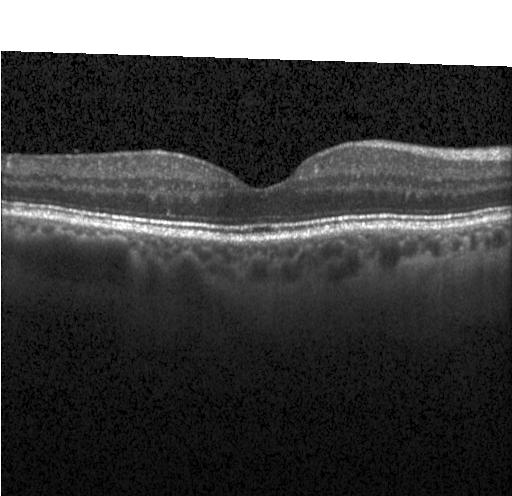

No evidence of CNV, DME, or drusen.